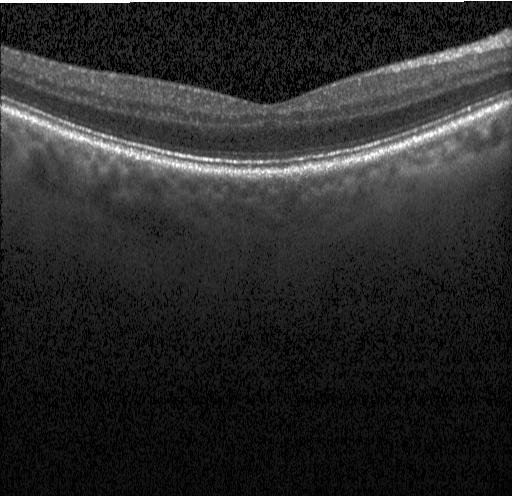

Impression: no CNV, DME, or drusen.